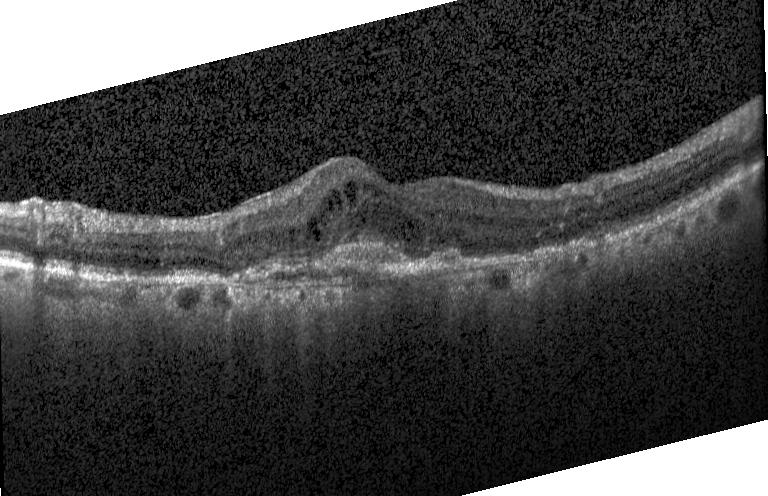 Optical coherence tomography scan
Macular OCT: choroidal neovascularization.